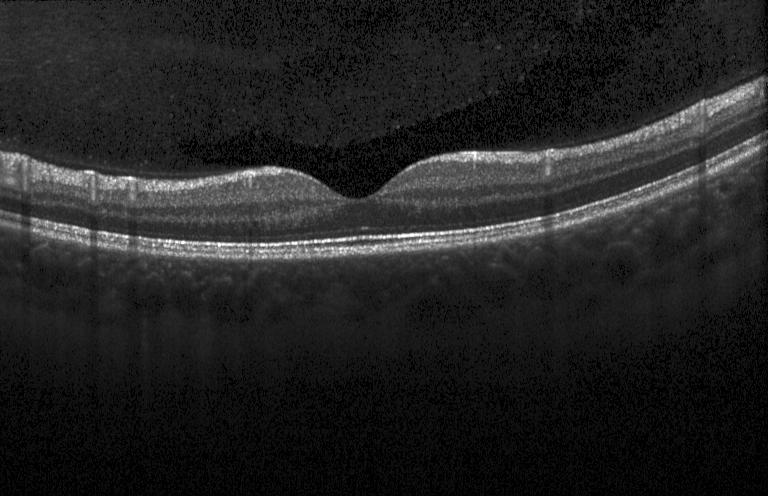

Centered on the fovea; instrument: Heidelberg Spectralis; optical coherence tomography B-scan.
Impression: no CNV, no DME, and no drusen.